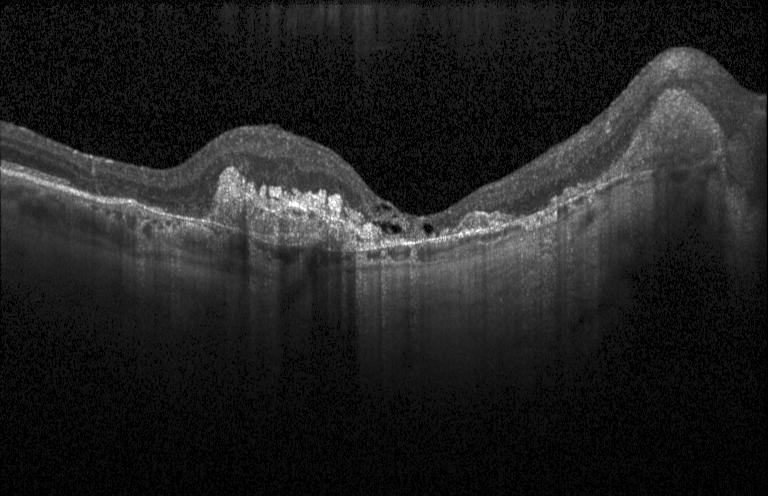 Retinal OCT B-scan.
Macular OCT: choroidal neovascularization.